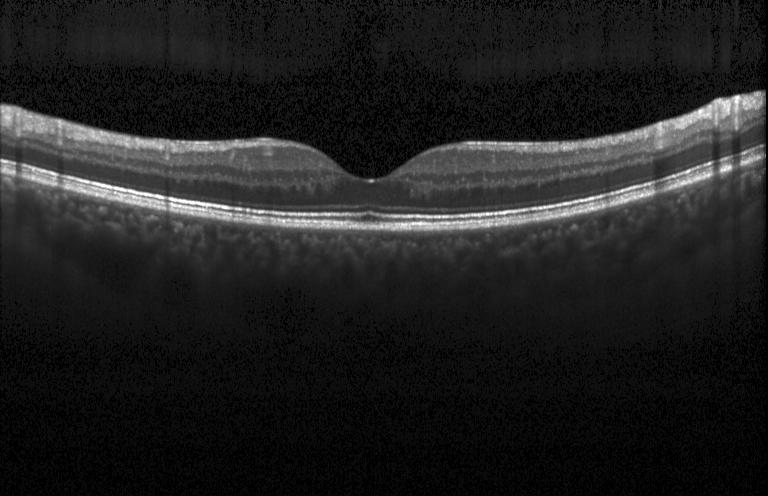

Retinal OCT B-scan. Impression: no evidence of CNV, DME, or drusen.